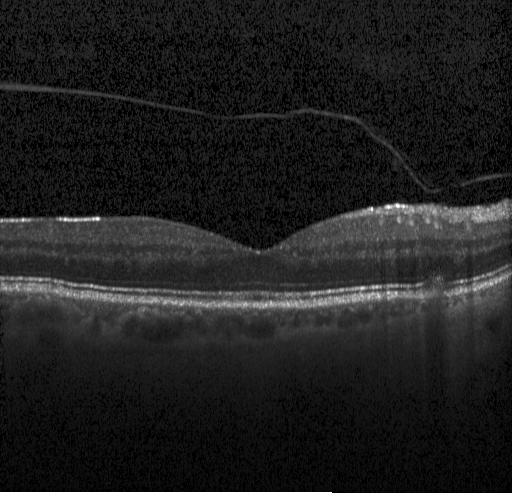 Heidelberg Spectralis OCT system, optical coherence tomography scan, spectral-domain optical coherence tomography, through the macula — Finding: no choroidal neovascularization, diabetic macular edema, or drusen.